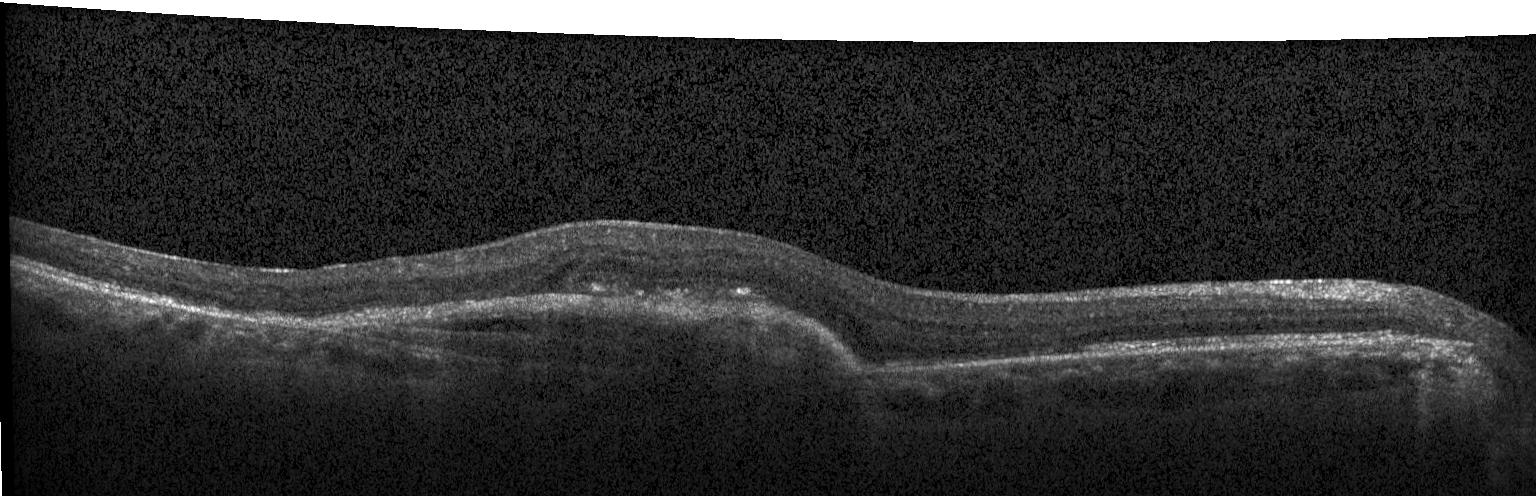

Dx: choroidal neovascularization (CNV).